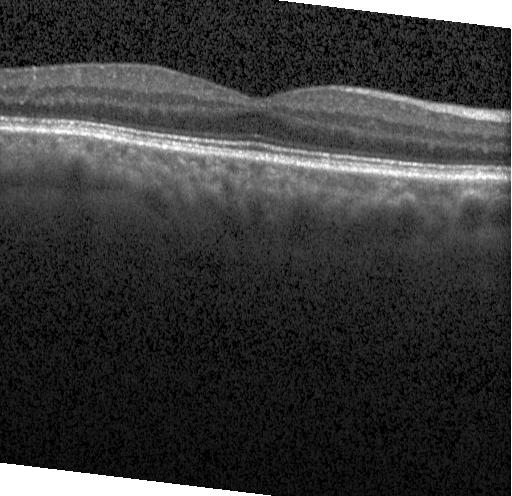

Retinal OCT B-scan
Impression: no CNV, no DME, and no drusen.